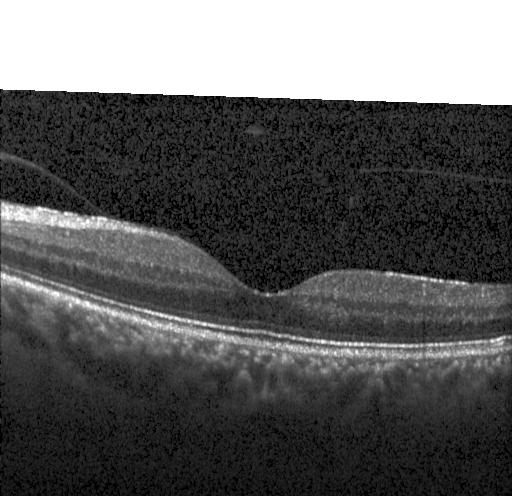

OCT finding: no evidence of choroidal neovascularization, diabetic macular edema, or drusen.